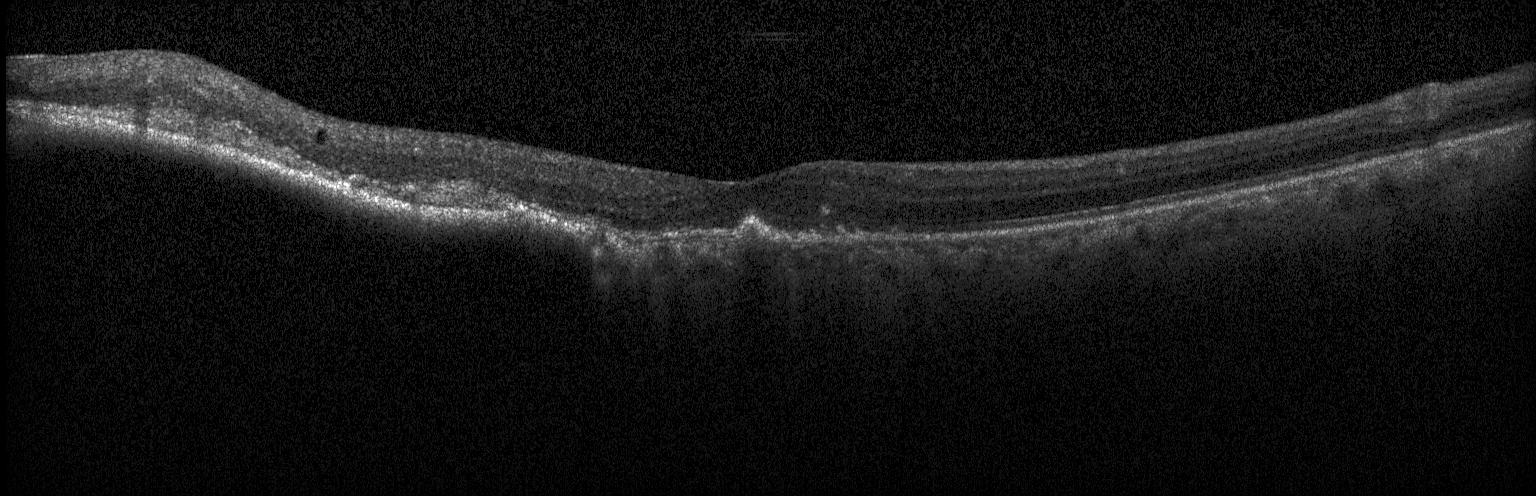
Macular OCT: a choroidal neovascular membrane.